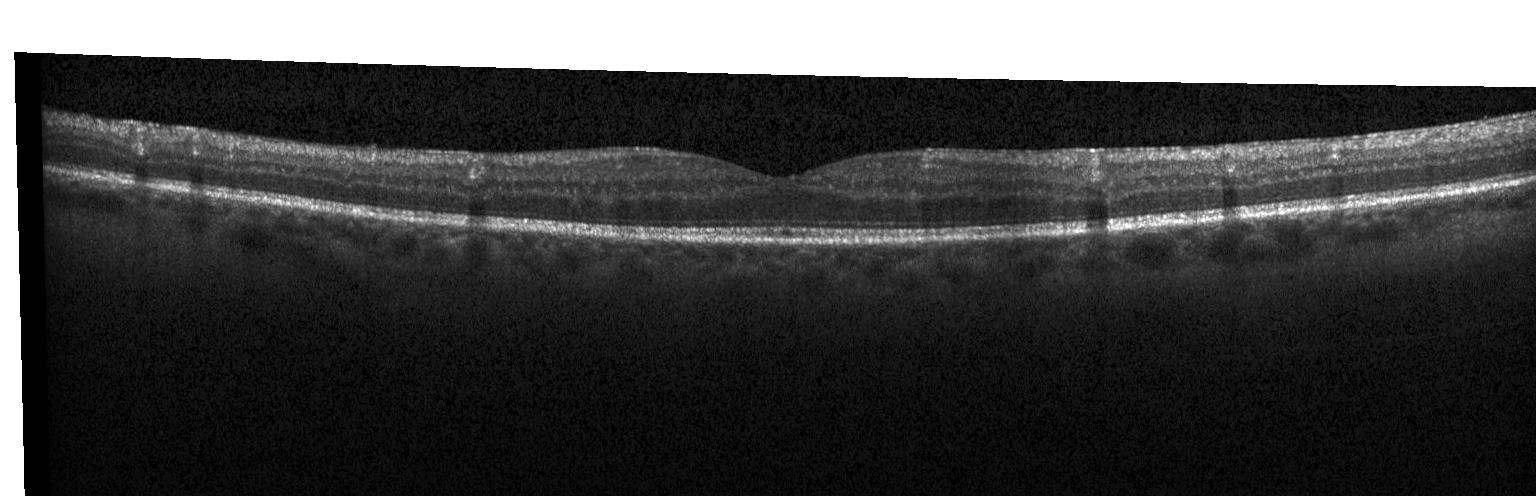 Fovea-centered. OCT B-scan. OCT finding: no evidence of choroidal neovascularization, diabetic macular edema, or drusen.